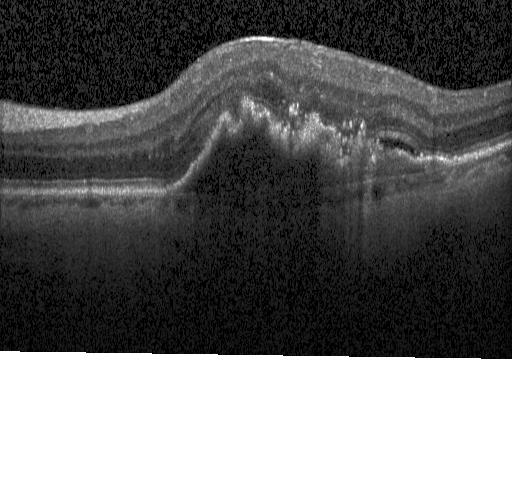
Optical coherence tomography scan. Spectral-domain optical coherence tomography. Fovea-centered. Heidelberg Spectralis.
Choroidal neovascularization (CNV).